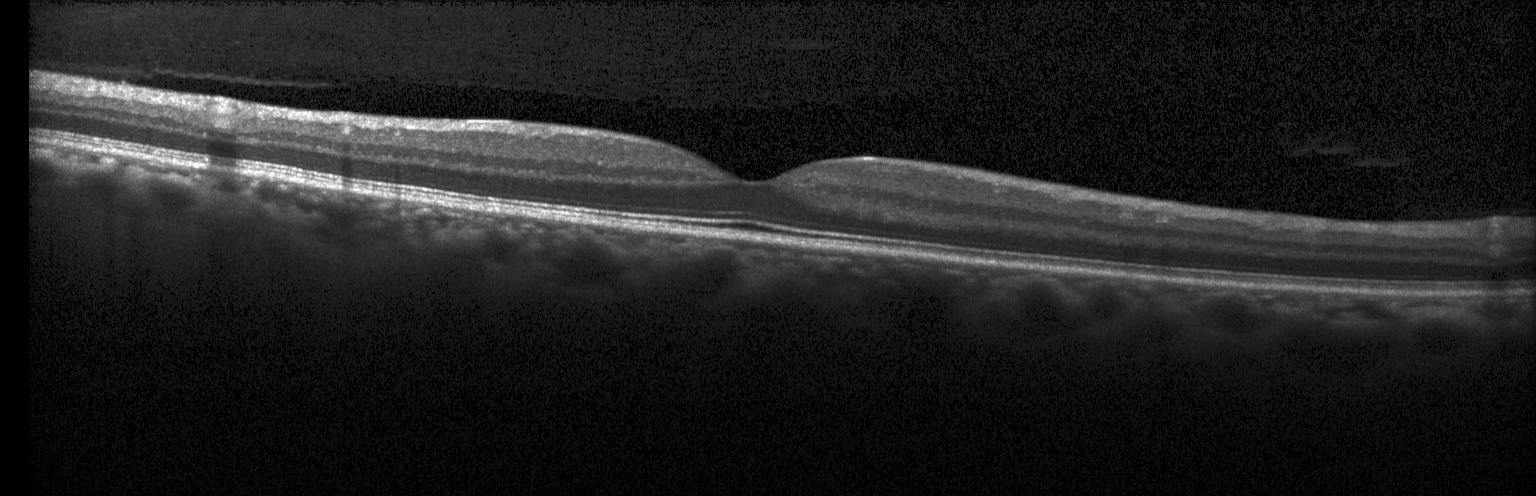 The scan shows no choroidal neovascularization, diabetic macular edema, or drusen.